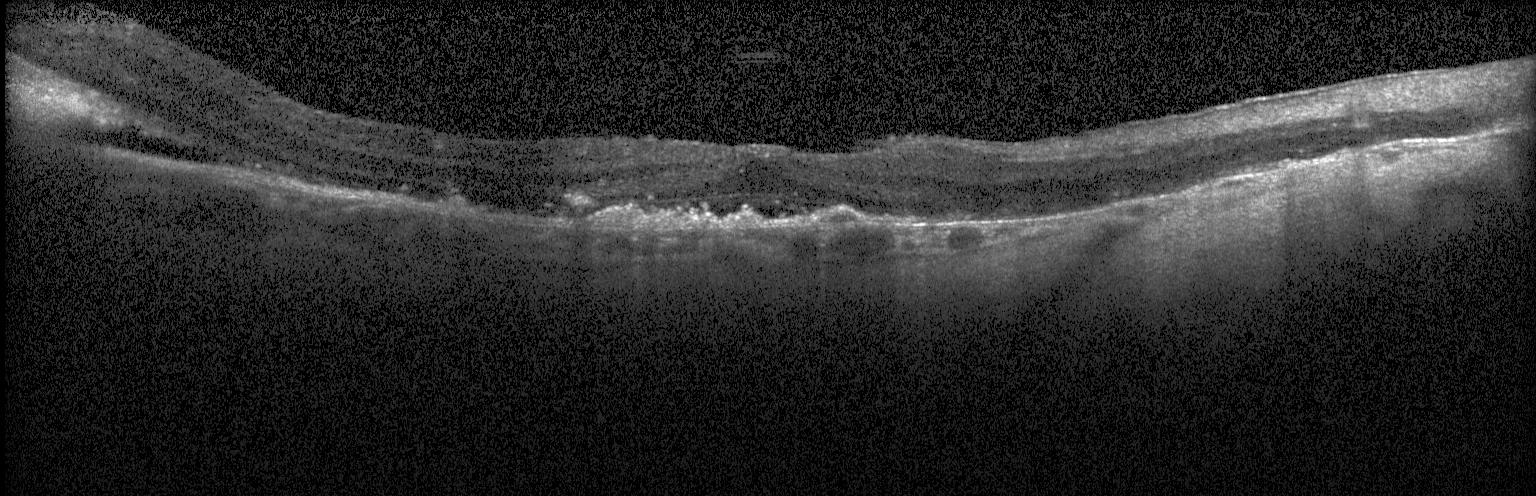
OCT line scan.
Macular OCT: choroidal neovascularization (CNV).